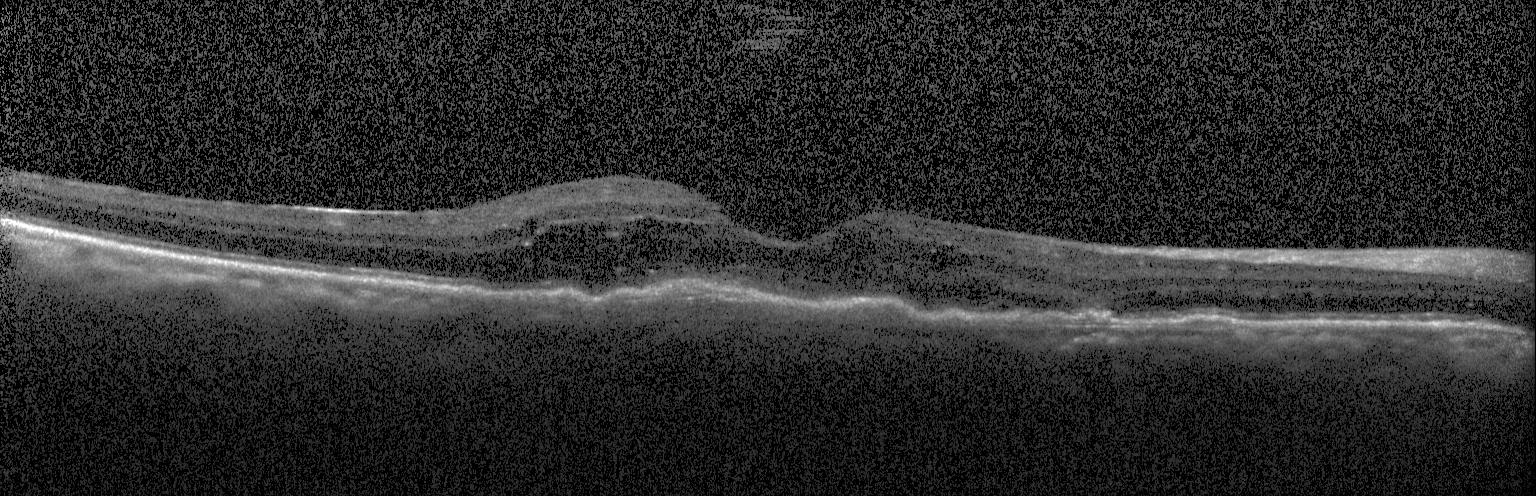
OCT finding: CNV.